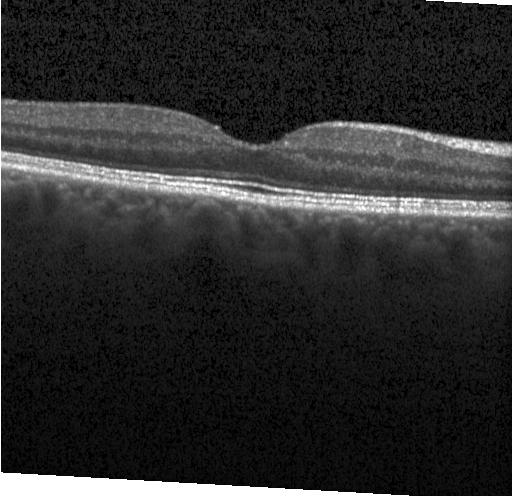
Impression: neither choroidal neovascularization, diabetic macular edema, nor drusen.